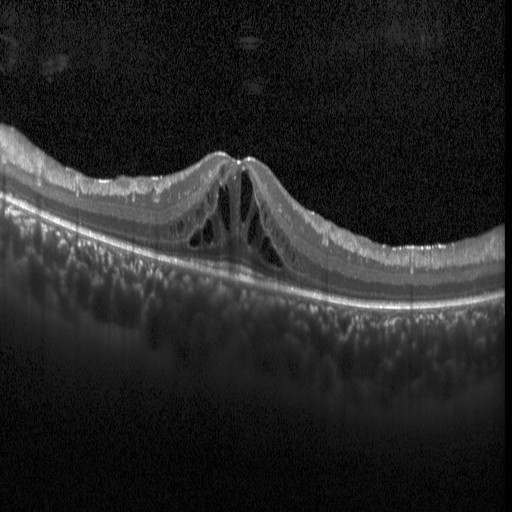 Diagnosis: DME.